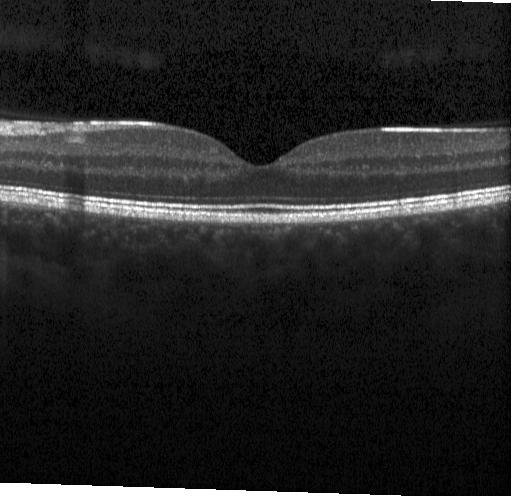

Optical coherence tomography B-scan; SD-OCT; acquired on a Heidelberg Spectralis; through the macula. Assessment: no CNV, DME, or drusen.